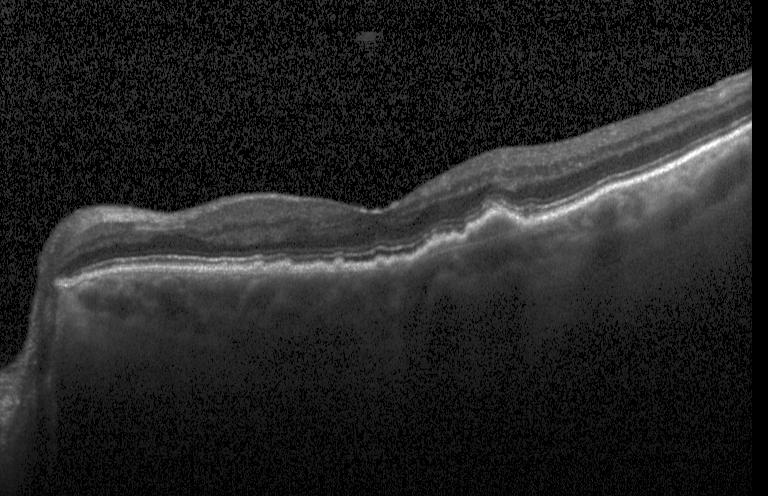
Spectral-domain OCT B-scan: choroidal neovascularization.